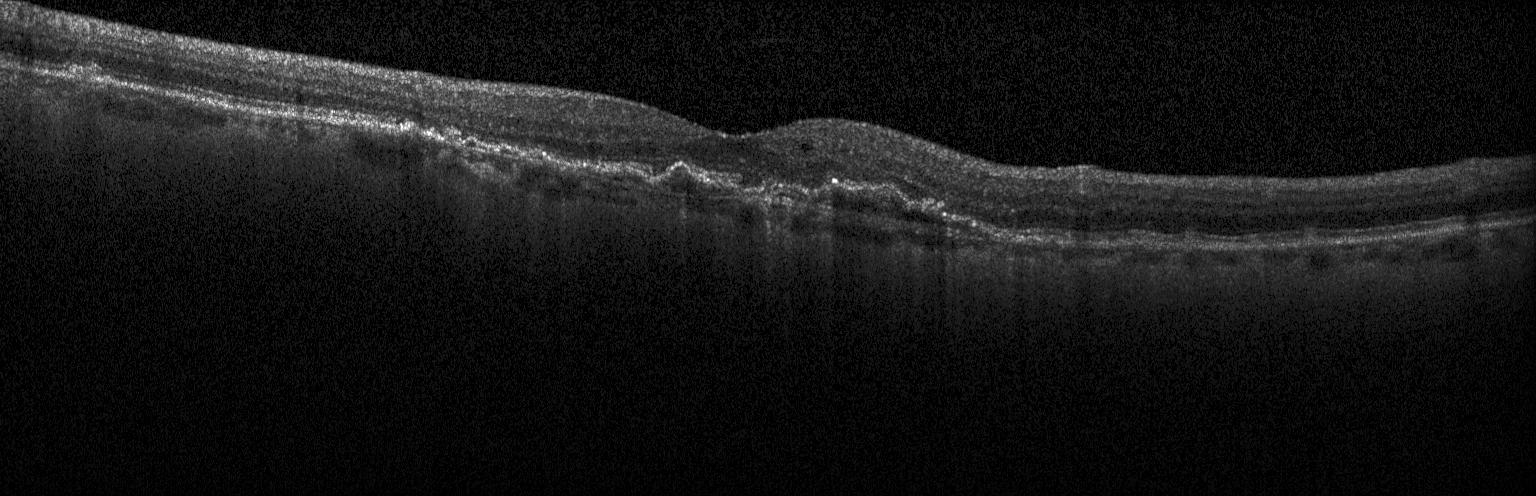

OCT line scan, Heidelberg Spectralis OCT system, SD-OCT
Finding: choroidal neovascularization (CNV).